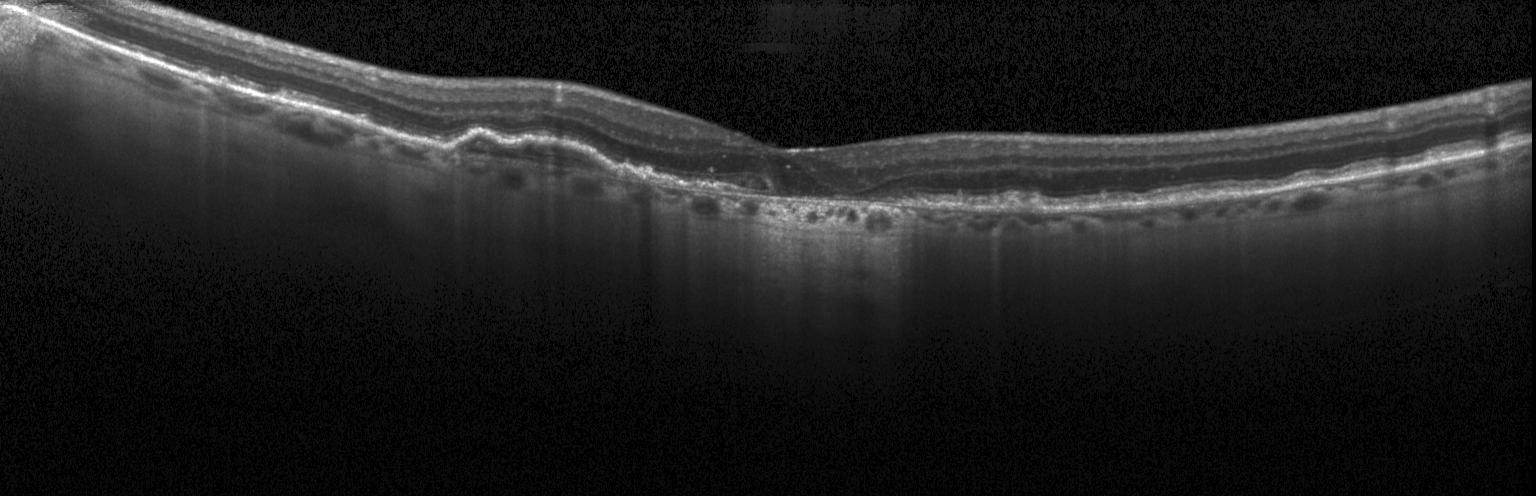
This B-scan demonstrates choroidal neovascularization.